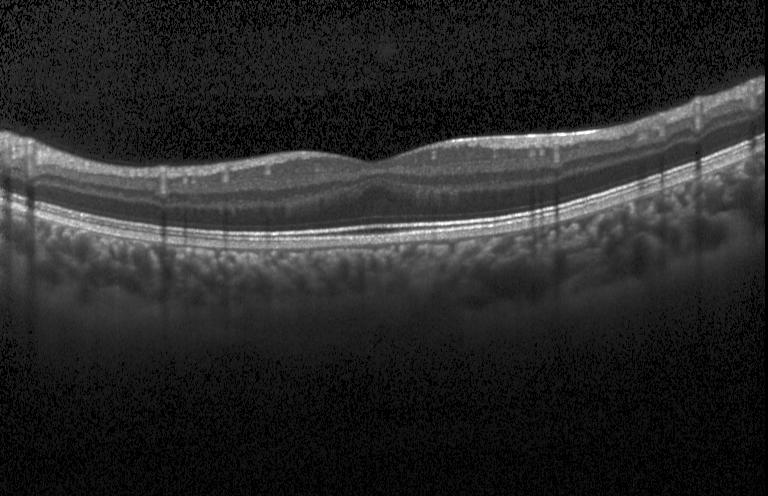 Retinal OCT cross-section showing no evidence of choroidal neovascularization, diabetic macular edema, or drusen.